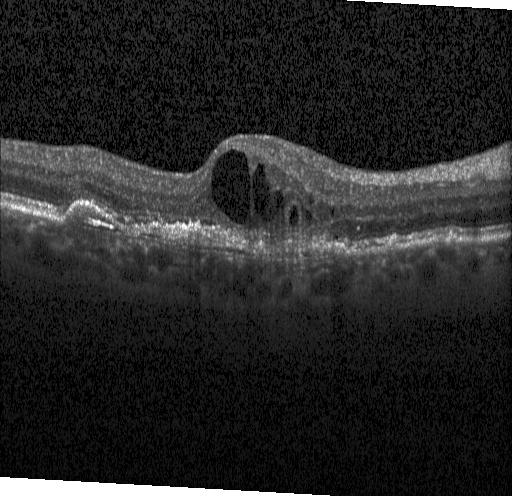

Impression: a choroidal neovascular membrane.